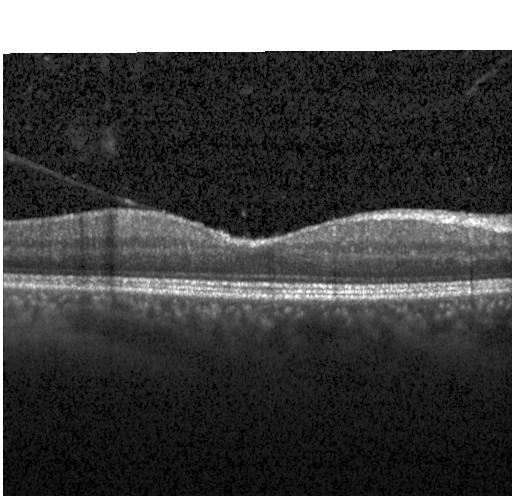

Finding: no choroidal neovascularization, diabetic macular edema, or drusen.